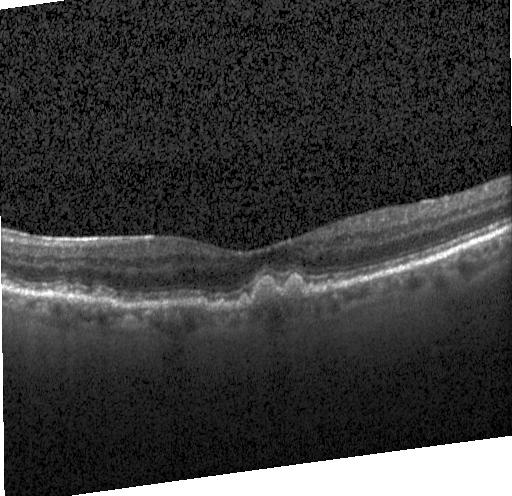
Impression: multiple drusen.